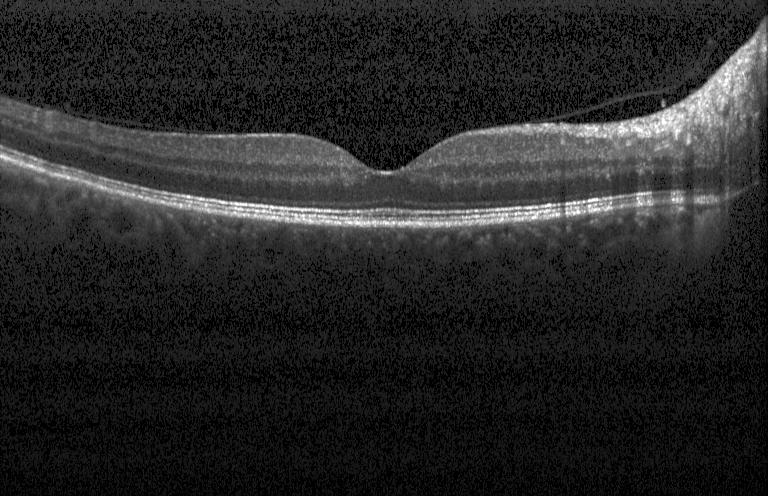

Through the macula, retinal OCT cross-section, spectral-domain OCT. Macular OCT: no choroidal neovascularization, no diabetic macular edema, and no drusen.